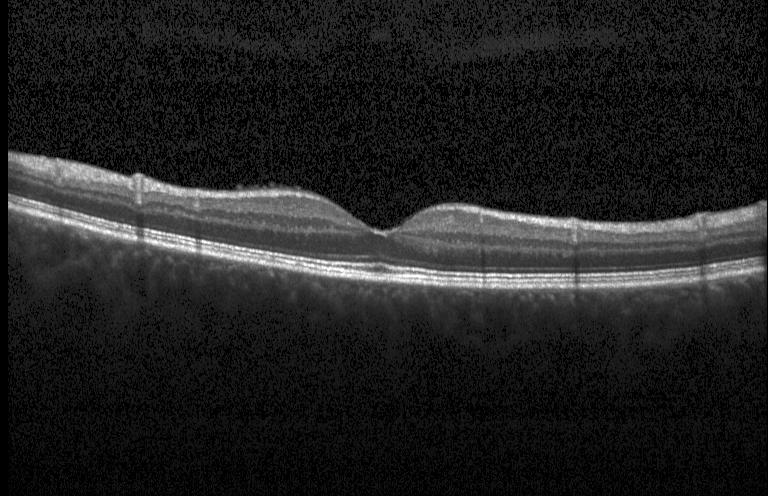
Macular scan; SD-OCT; OCT B-scan
This B-scan demonstrates no choroidal neovascularization, diabetic macular edema, or drusen.